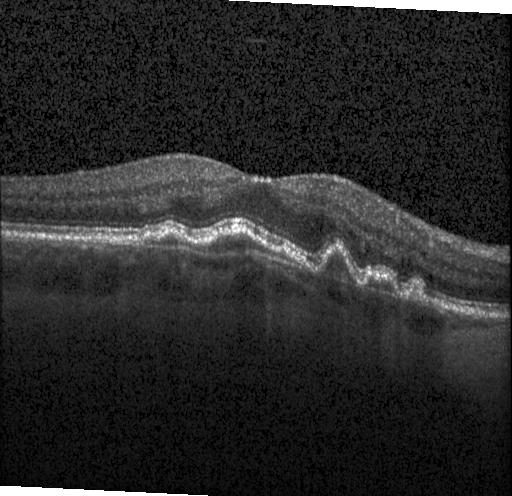

OCT B-scan — Diagnosis: choroidal neovascularization.